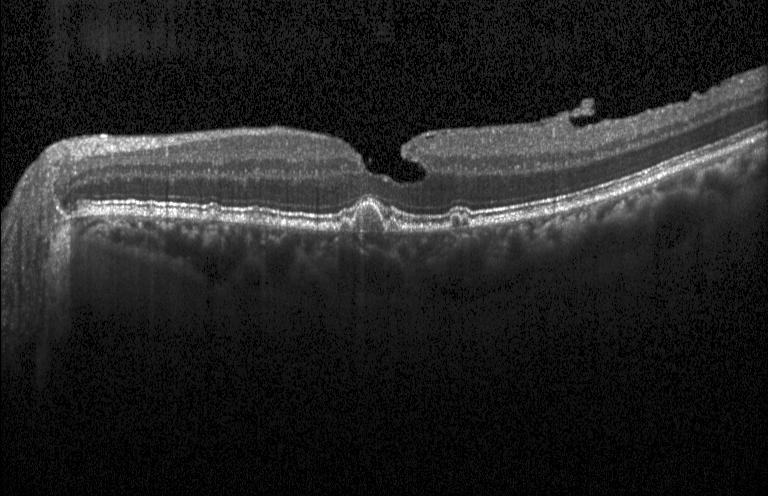

OCT B-scan · macular scan · acquired on a Heidelberg Spectralis · spectral-domain optical coherence tomography
Macular OCT: sub-RPE drusenoid deposits.